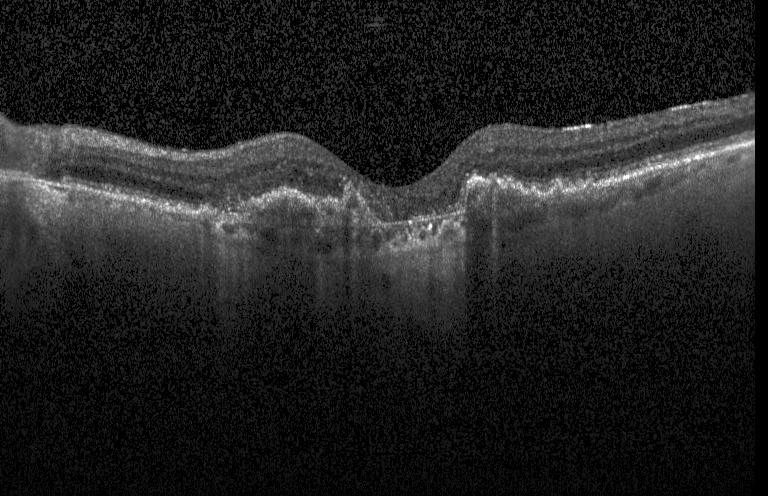
Macular OCT demonstrating a choroidal neovascular membrane.